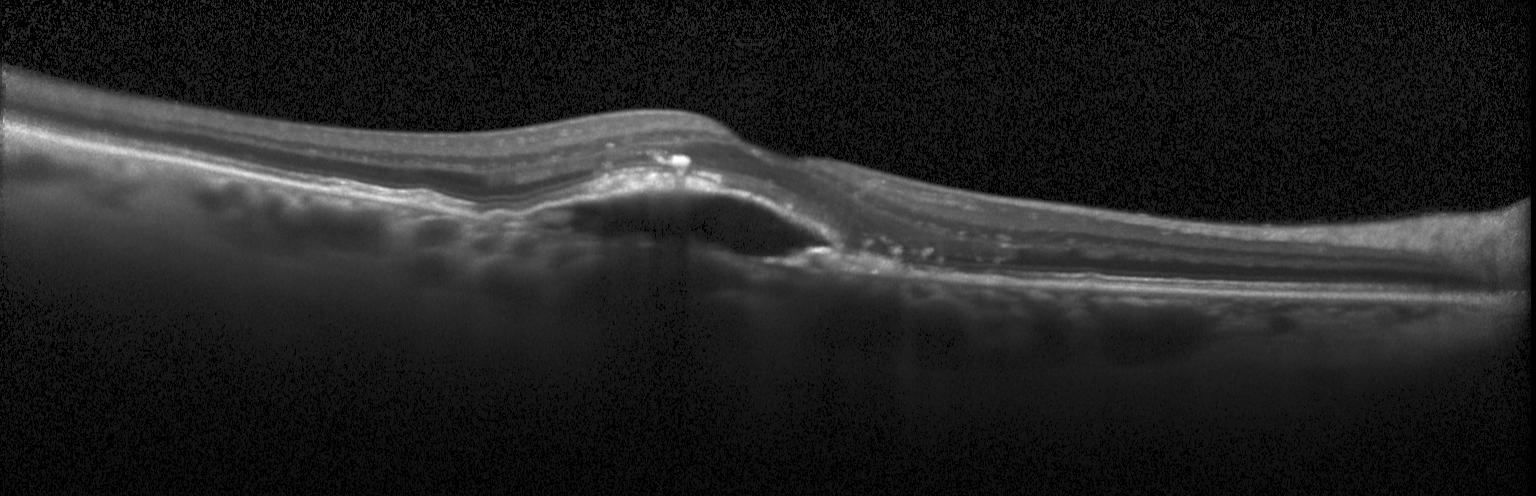
Centered on the fovea · OCT B-scan · Heidelberg Spectralis OCT system · SD-OCT — OCT finding: a choroidal neovascular membrane.